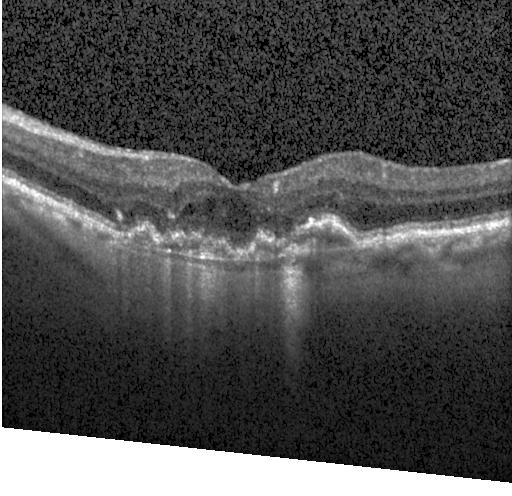

OCT finding: a choroidal neovascular membrane.